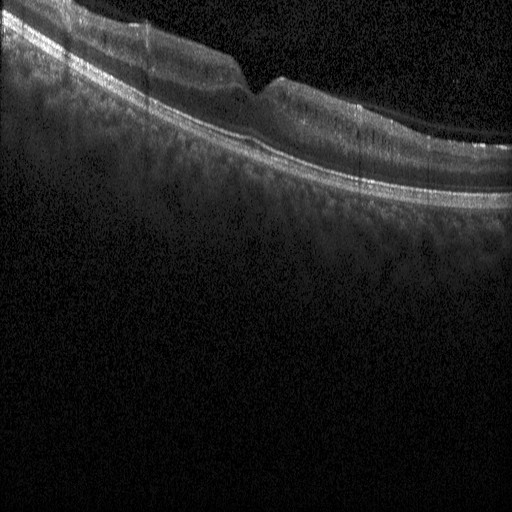
SD-OCT, macular scan, optical coherence tomography scan, acquired on a Heidelberg Spectralis — Assessment: DME.